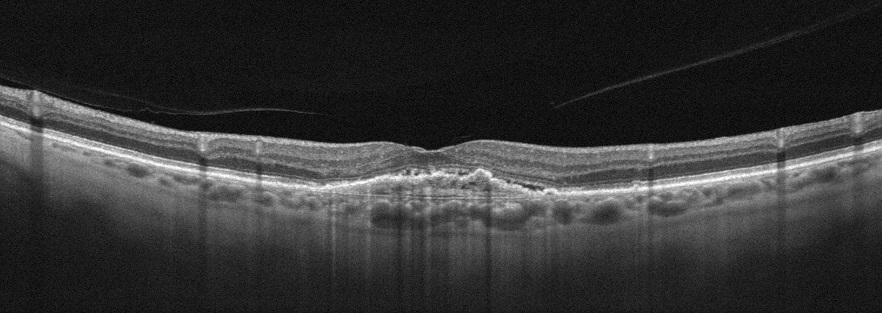
OCT line scan.
This B-scan demonstrates age-related macular degeneration (AMD).